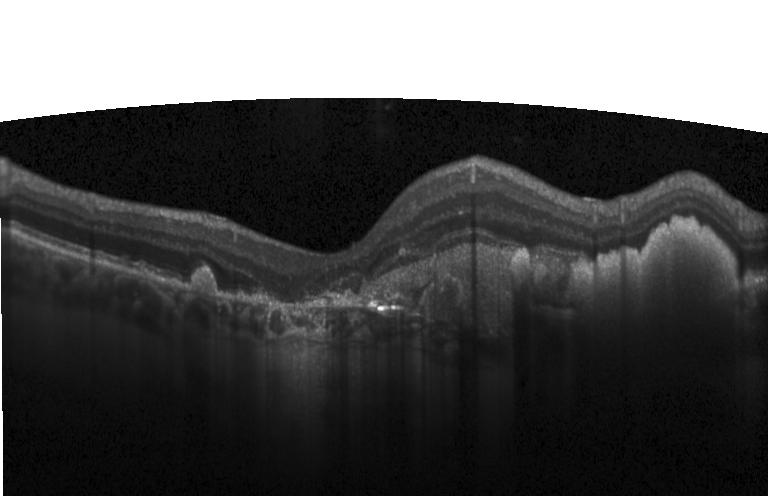

Spectral-domain optical coherence tomography. Heidelberg Spectralis OCT system. Through the macula. Retinal OCT cross-section — This B-scan demonstrates CNV.